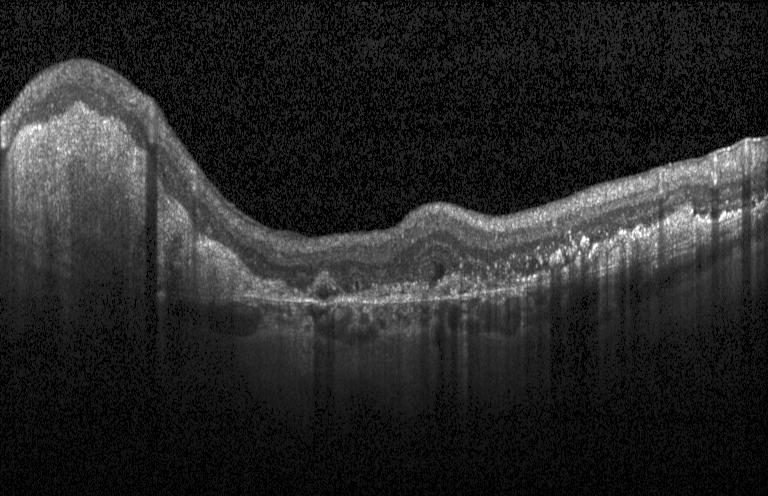

Retinal OCT cross-section — The scan shows a choroidal neovascular membrane.